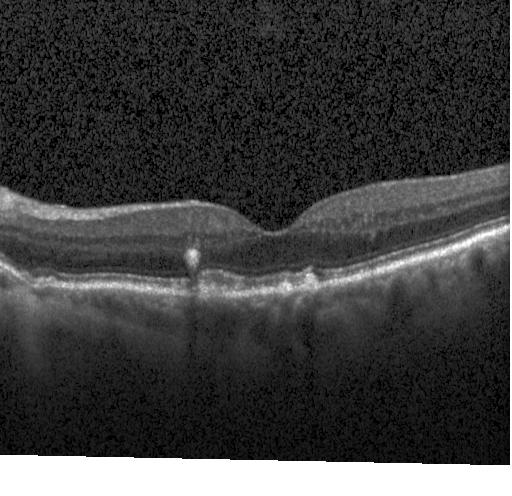 Through the macula. OCT B-scan. Instrument: Heidelberg Spectralis. Spectral-domain OCT. The scan shows drusen.